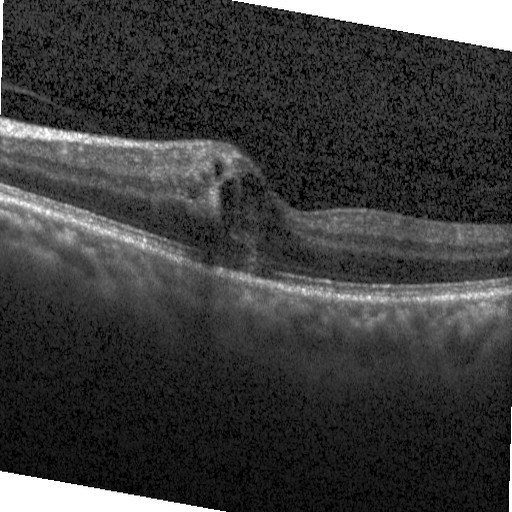
Retinal OCT B-scan; acquired on a Heidelberg Spectralis
Macular OCT: diabetic macular edema.